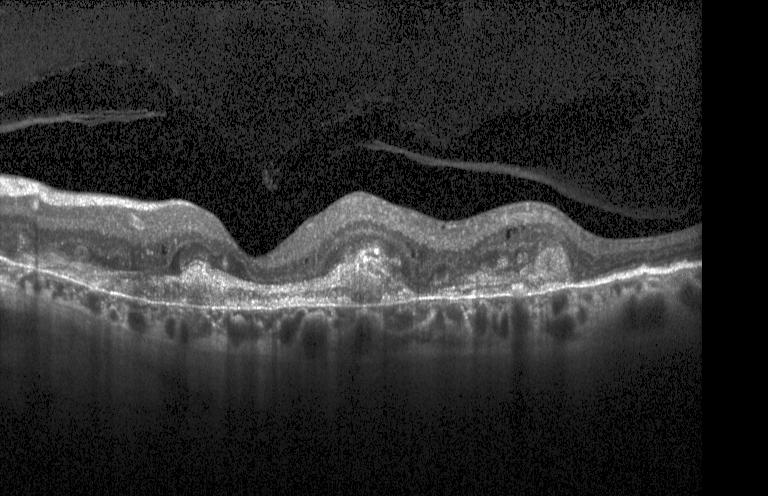 Finding: a choroidal neovascular membrane.